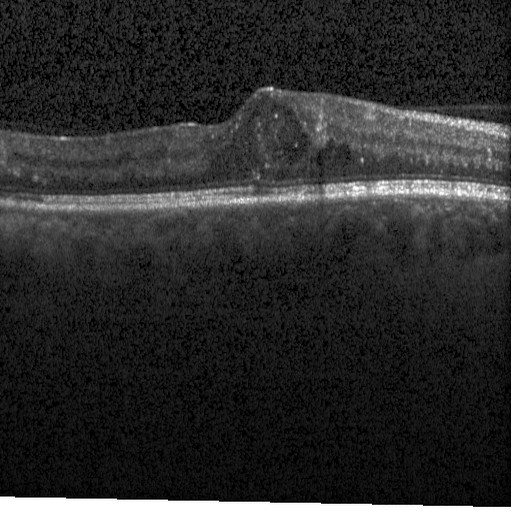

The scan shows diabetic macular edema.